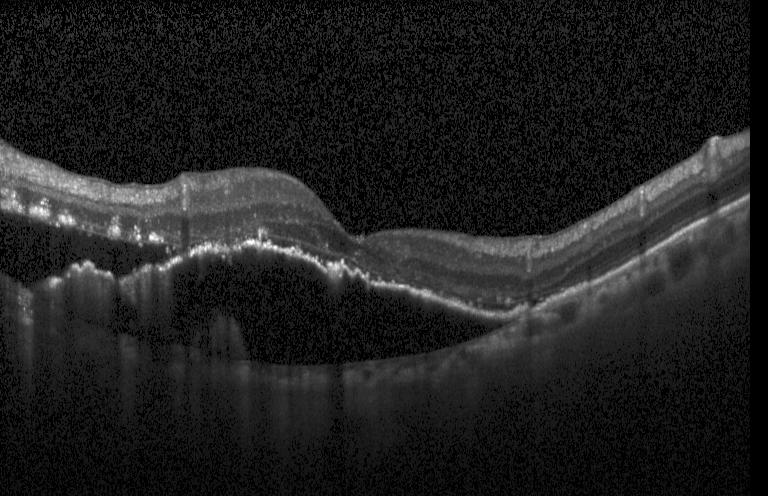 Finding: a choroidal neovascular membrane.